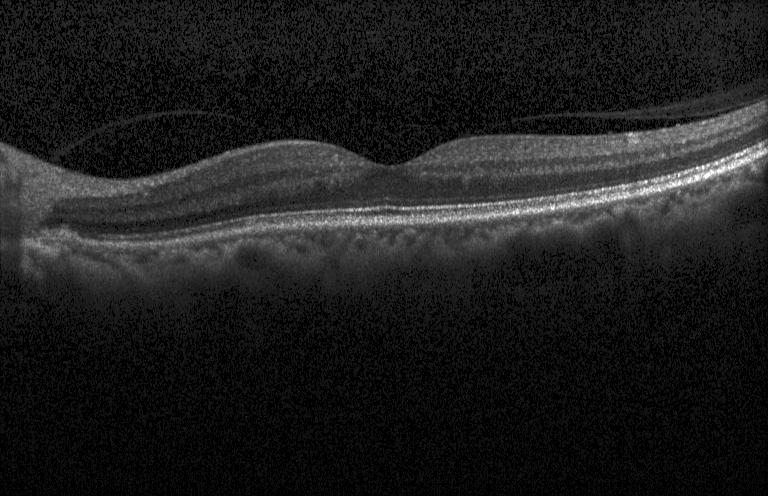

Instrument: Heidelberg Spectralis · macular scan · spectral-domain optical coherence tomography · optical coherence tomography B-scan.
Finding: no choroidal neovascularization, diabetic macular edema, or drusen.